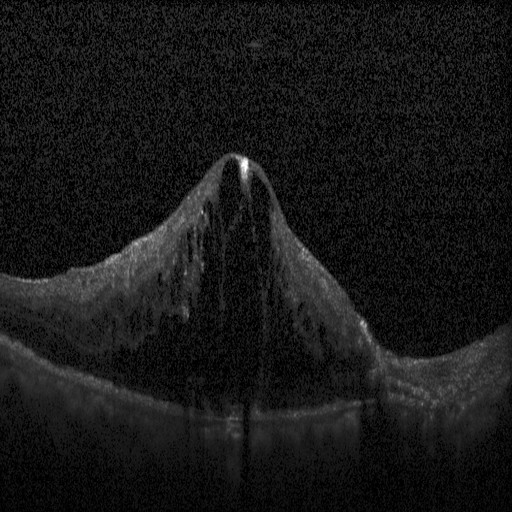

This B-scan demonstrates DME.